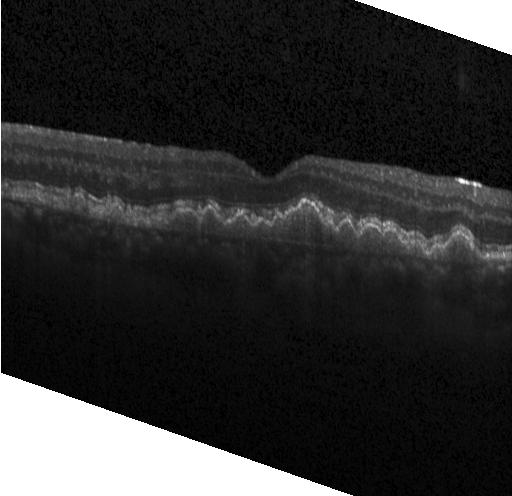
Retinal OCT cross-section
Finding: choroidal neovascularization (CNV).